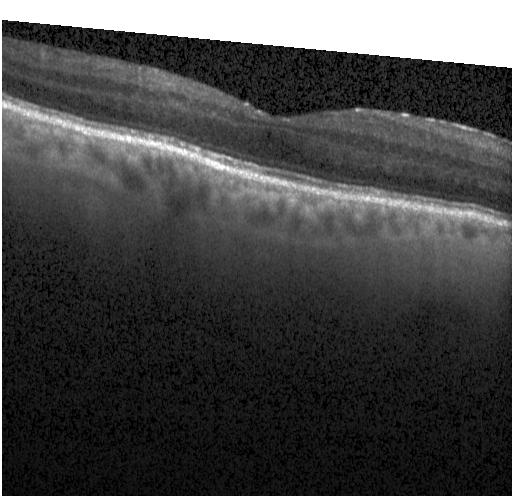 Retinal OCT cross-section showing no choroidal neovascularization, diabetic macular edema, or drusen.